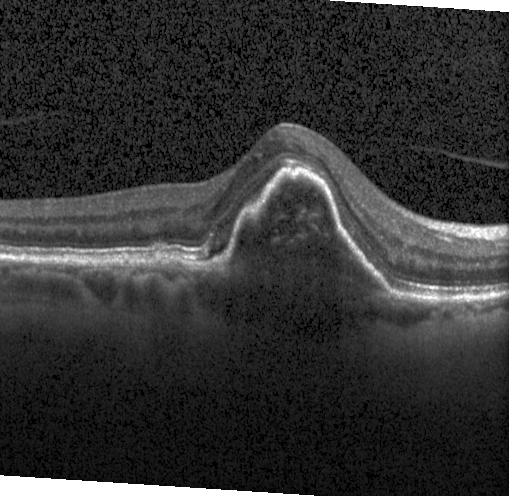

Optical coherence tomography B-scan. Macular OCT: a choroidal neovascular membrane.